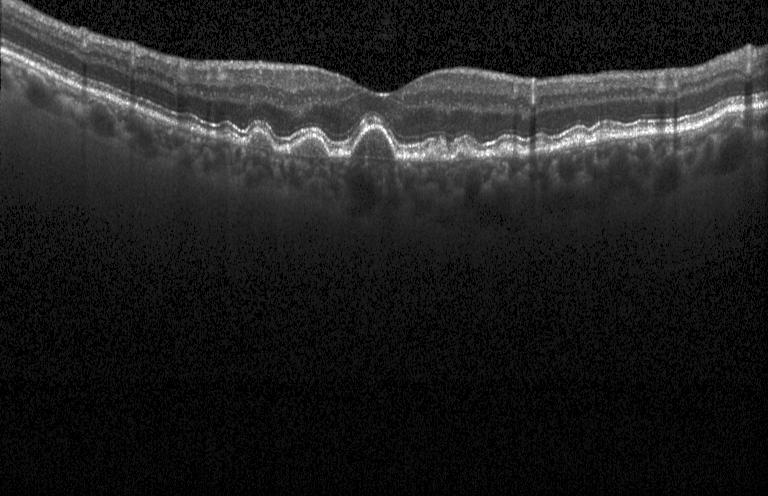

OCT scan showing multiple drusen.